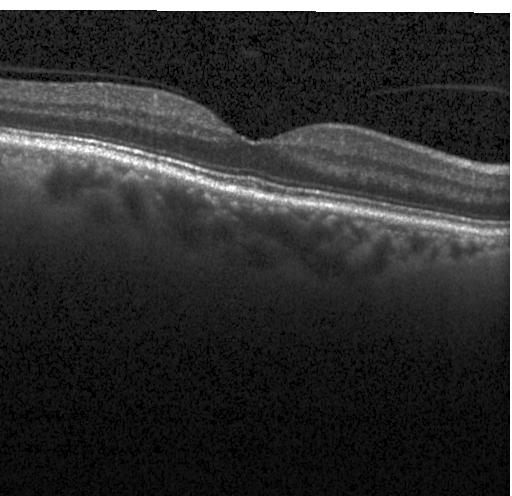

OCT line scan
Finding: neither choroidal neovascularization, diabetic macular edema, nor drusen.